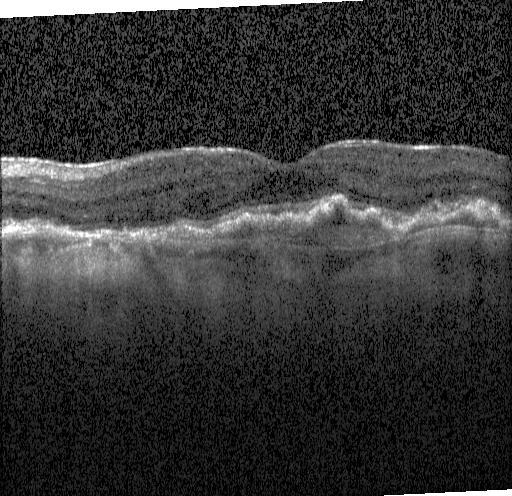 Finding: a choroidal neovascular membrane.